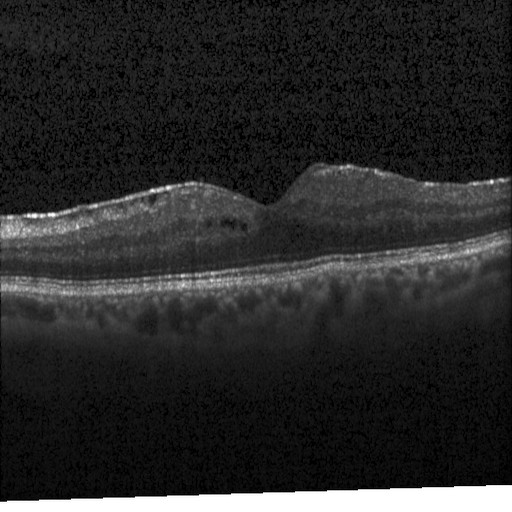

The scan shows diabetic macular edema.